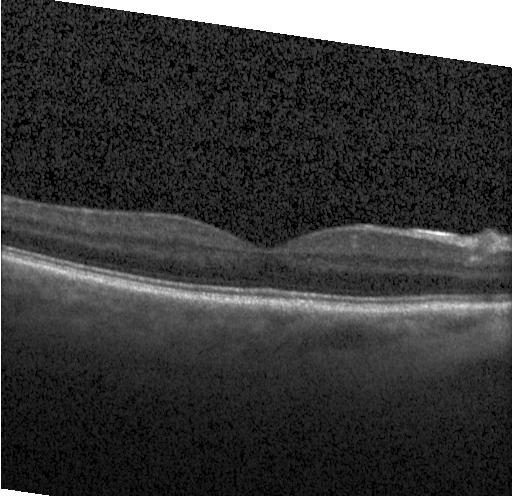
This B-scan demonstrates no evidence of CNV, DME, or drusen.